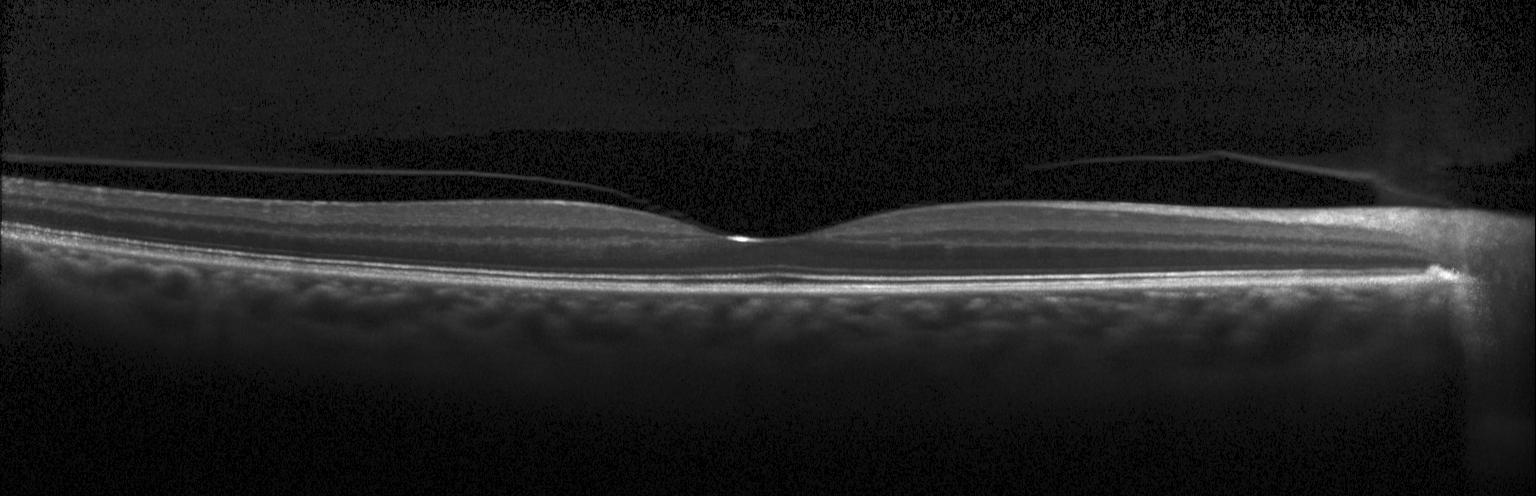 Retinal OCT cross-section, spectral-domain optical coherence tomography, acquired on a Heidelberg Spectralis
OCT finding: neither choroidal neovascularization, diabetic macular edema, nor drusen.